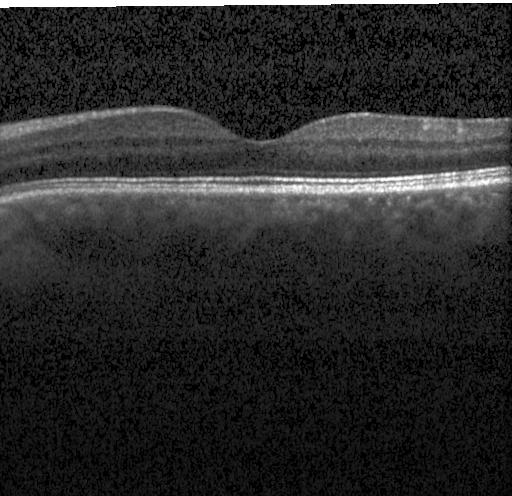
Impression: neither choroidal neovascularization, diabetic macular edema, nor drusen.